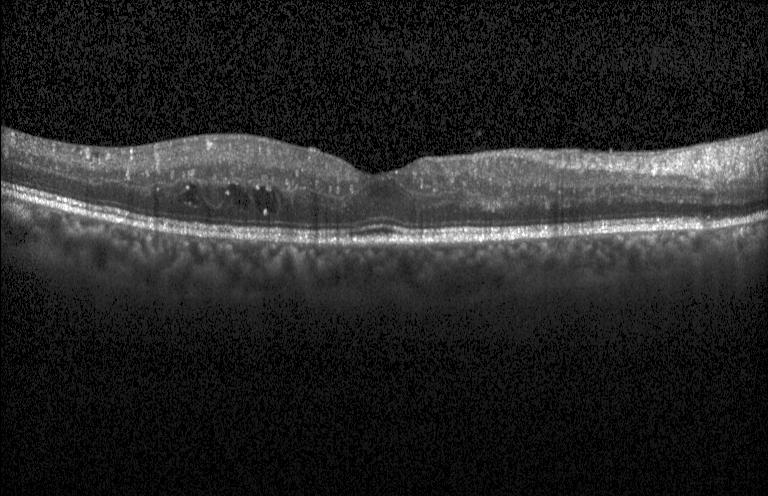 Retinal OCT cross-section
Impression: DME.